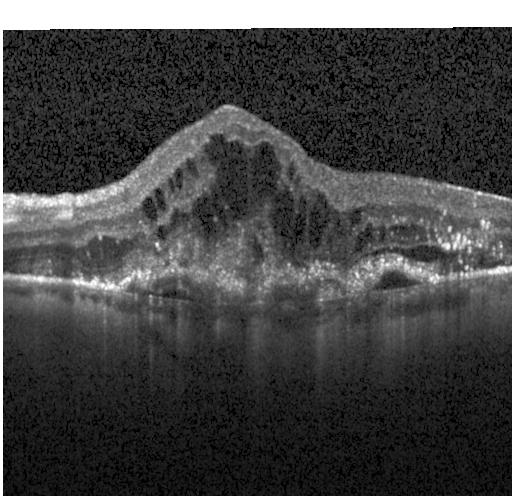
A choroidal neovascular membrane.